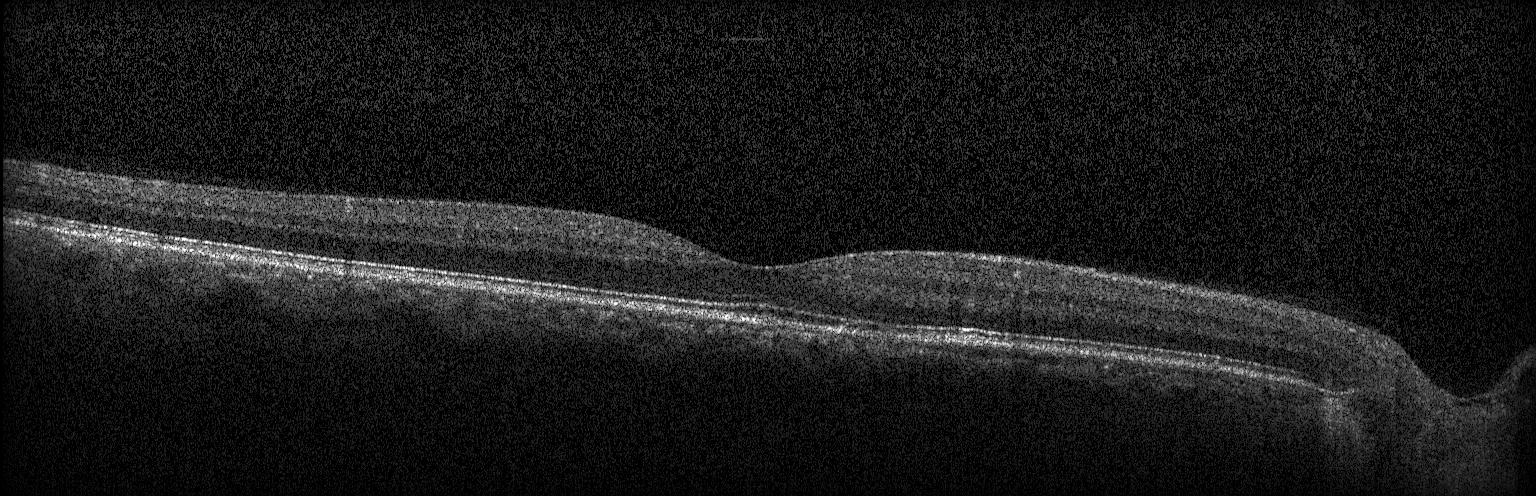
Acquired on a Heidelberg Spectralis · optical coherence tomography B-scan · spectral-domain optical coherence tomography — Finding: neither choroidal neovascularization, diabetic macular edema, nor drusen.